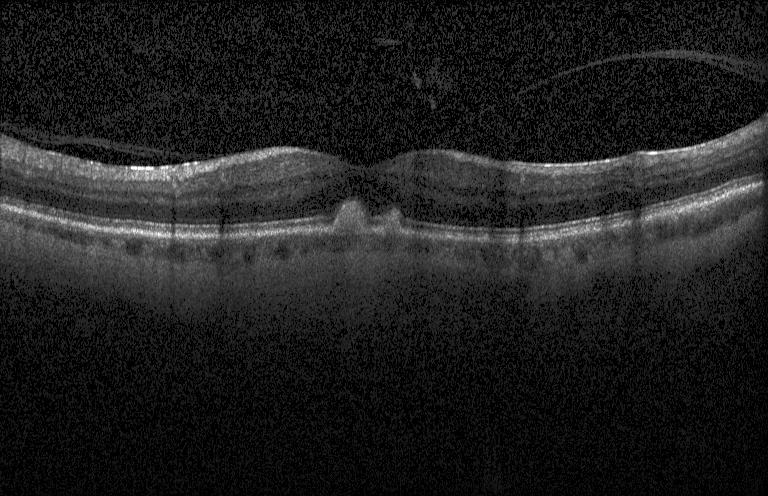
Retinal OCT B-scan · through the macula · Heidelberg Spectralis OCT system · spectral-domain optical coherence tomography
OCT finding: multiple drusen.